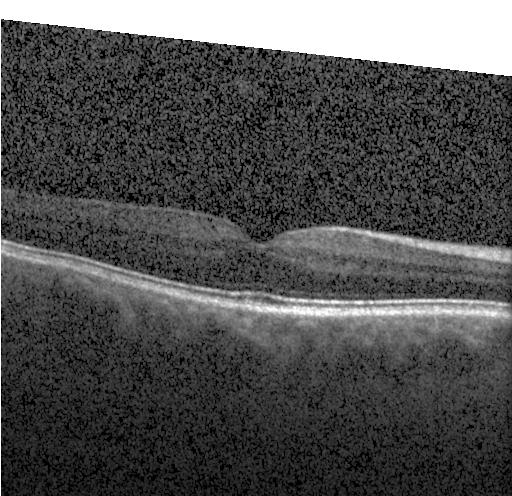

Dx: no CNV, no DME, and no drusen.